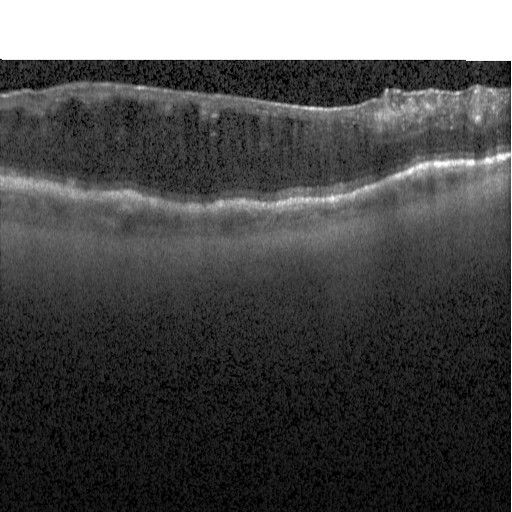 Spectral-domain OCT. Macular scan. OCT line scan.
This B-scan demonstrates diabetic macular edema.